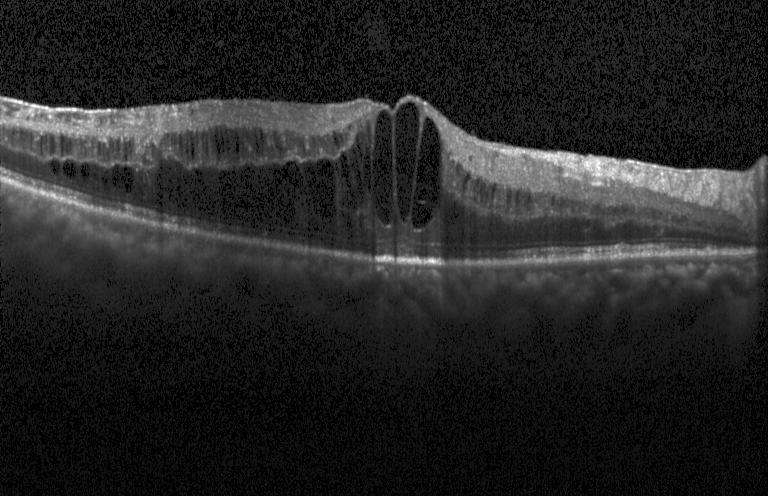
Macular OCT: DME.